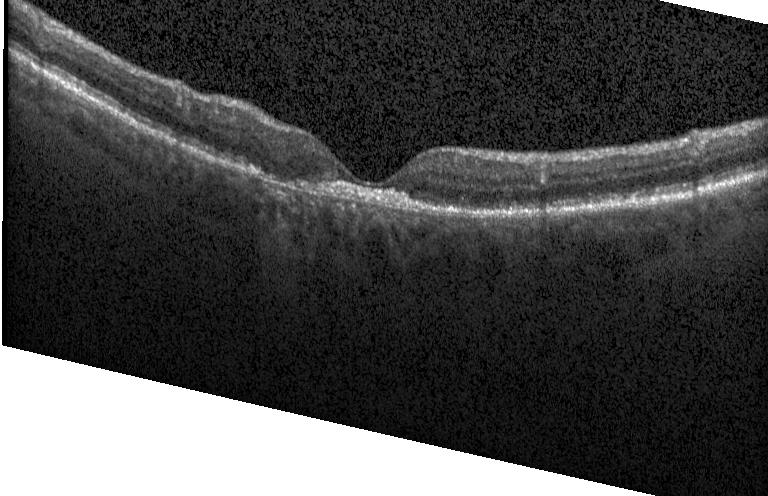

Centered on the fovea · acquired on a Heidelberg Spectralis · optical coherence tomography B-scan · spectral-domain optical coherence tomography. Impression: choroidal neovascularization.